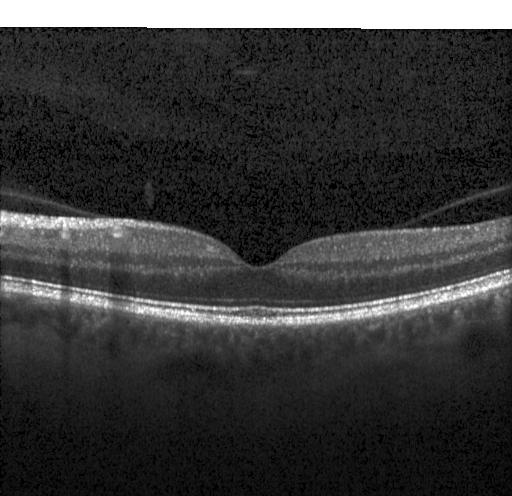

Through the macula, instrument: Heidelberg Spectralis, retinal OCT cross-section, spectral-domain OCT
This B-scan demonstrates no evidence of choroidal neovascularization, diabetic macular edema, or drusen.